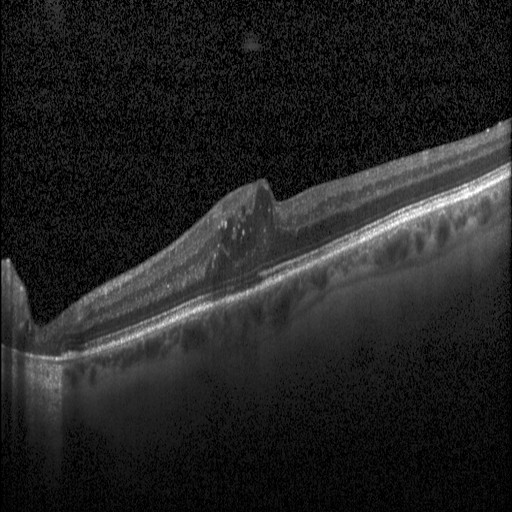
Finding: diabetic macular edema.